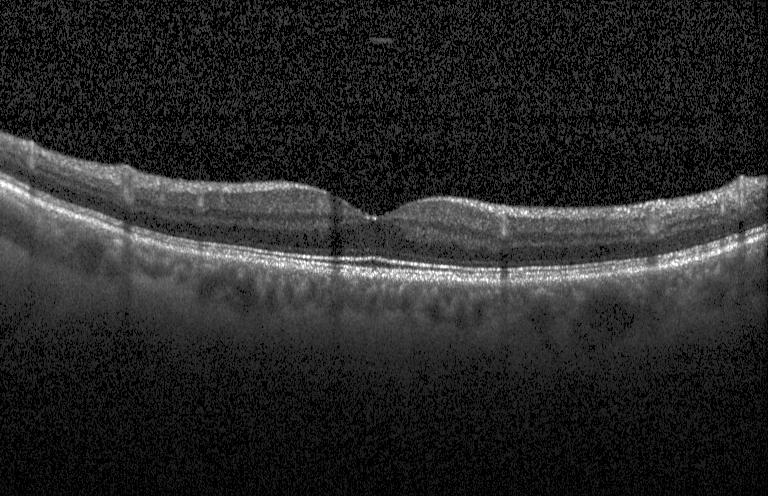
Heidelberg Spectralis OCT system, retinal OCT cross-section. Diagnosis: neither choroidal neovascularization, diabetic macular edema, nor drusen.